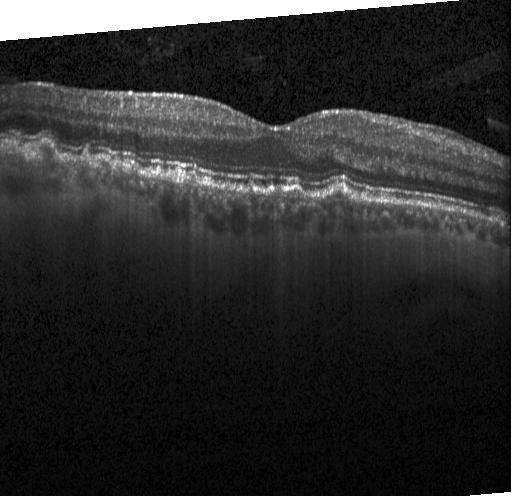

Retinal OCT cross-section · through the macula — OCT finding: multiple drusen.